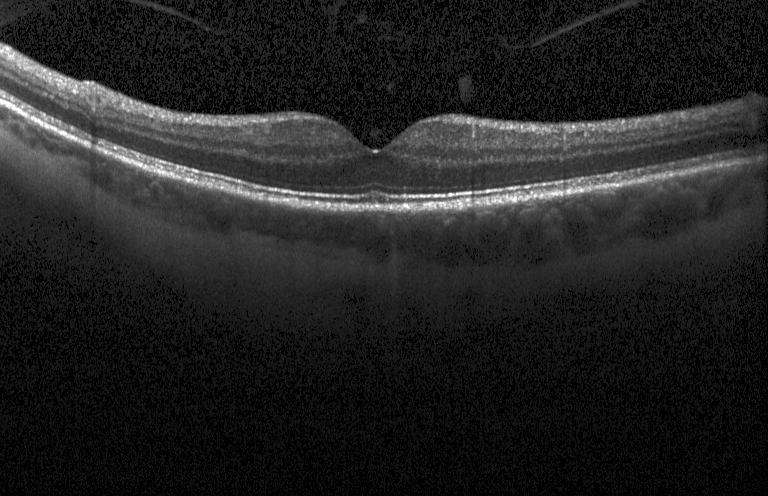 OCT B-scan — Macular OCT: no choroidal neovascularization, no diabetic macular edema, and no drusen.